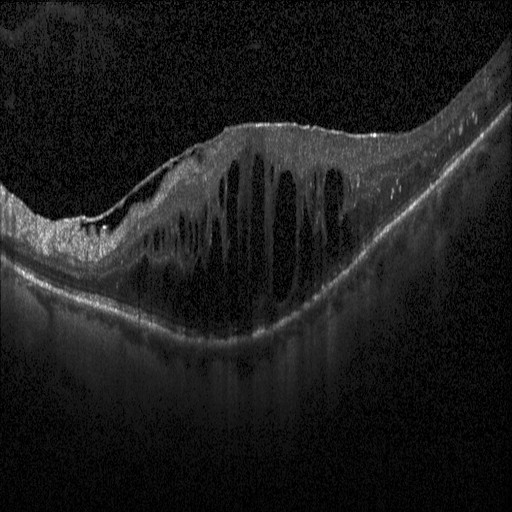
Macular scan; retinal OCT cross-section — OCT finding: diabetic macular edema (DME).